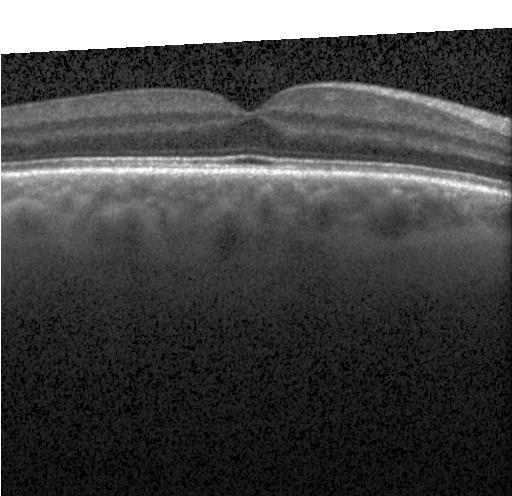
Through the macula; optical coherence tomography scan; instrument: Heidelberg Spectralis.
No CNV, DME, or drusen.